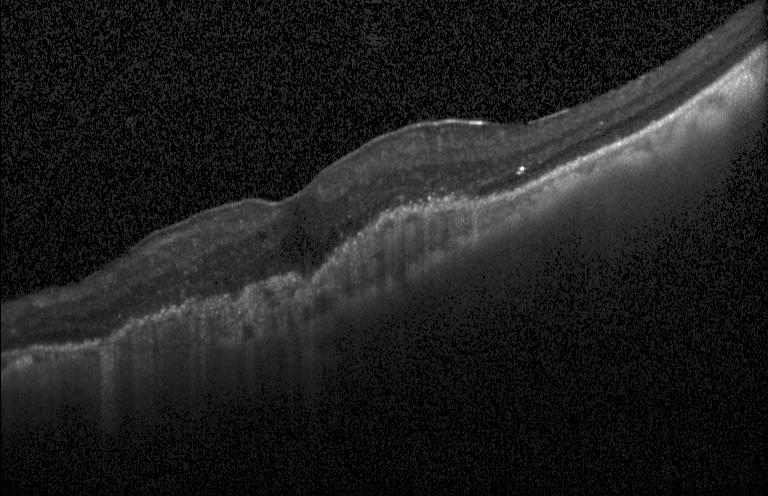

Heidelberg Spectralis OCT system · SD-OCT · optical coherence tomography scan · horizontal scan through the fovea. Diagnosis: choroidal neovascularization (CNV).